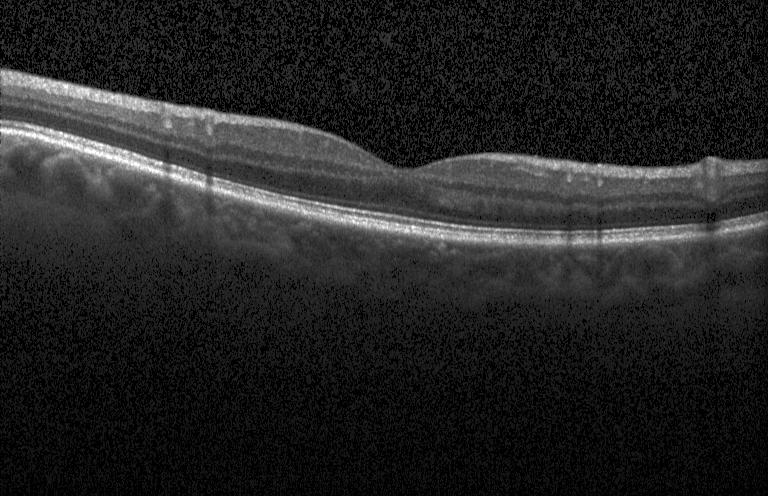 No evidence of CNV, DME, or drusen.